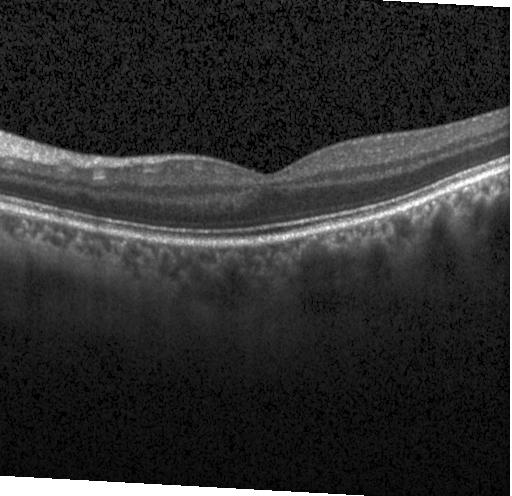

Spectral-domain OCT · OCT B-scan.
Diagnosis: neither CNV, DME, nor drusen.